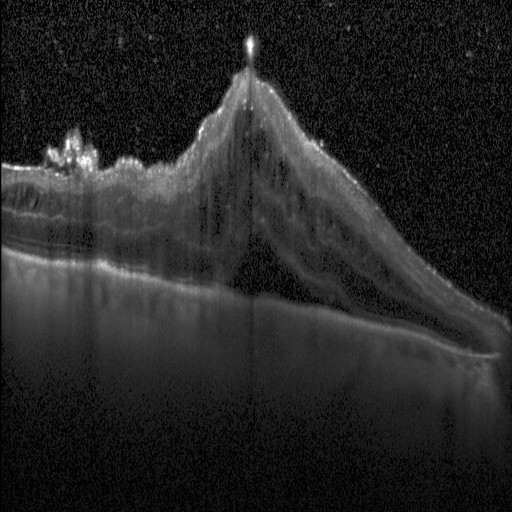
The scan shows diabetic macular edema.